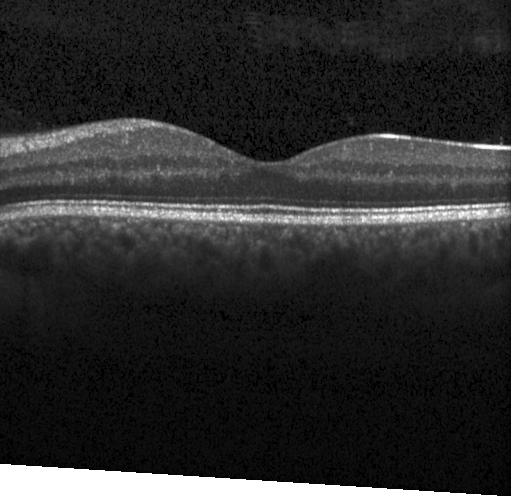 Optical coherence tomography B-scan. Macular OCT: neither choroidal neovascularization, diabetic macular edema, nor drusen.